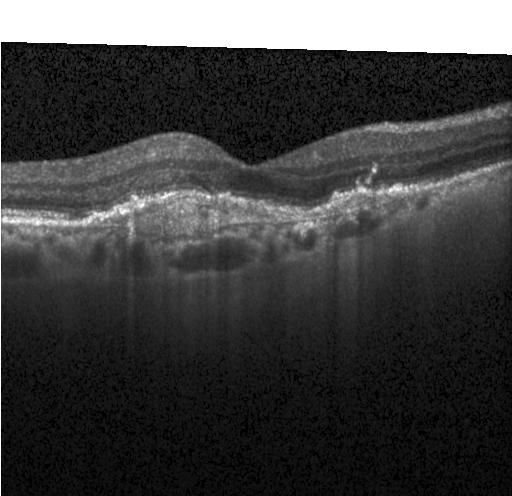
OCT B-scan, spectral-domain OCT.
Finding: choroidal neovascularization (CNV).